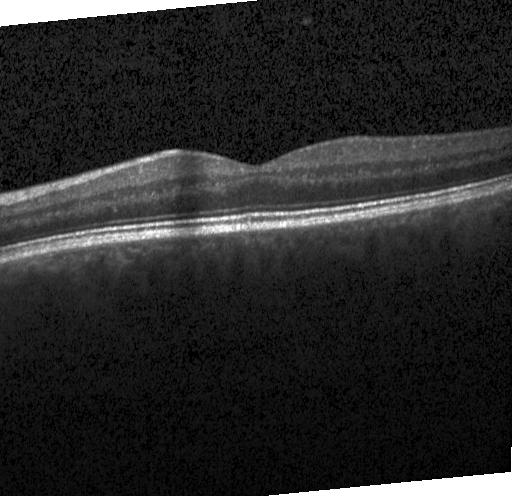

OCT scan showing neither choroidal neovascularization, diabetic macular edema, nor drusen.